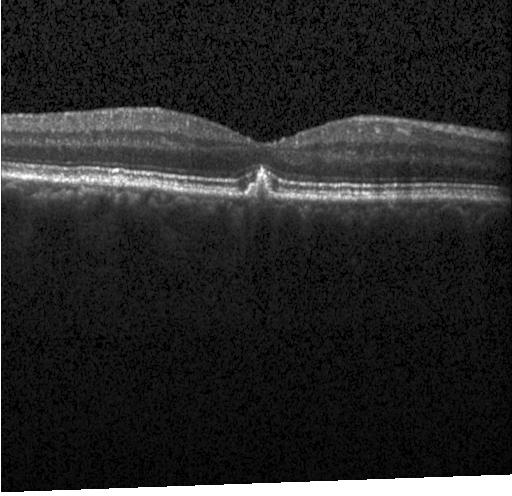 Spectral-domain OCT B-scan: sub-RPE drusenoid deposits.